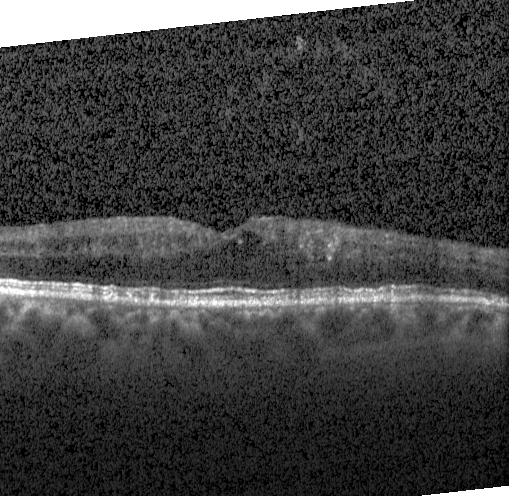 Macular scan · optical coherence tomography scan — Diagnosis: DME.